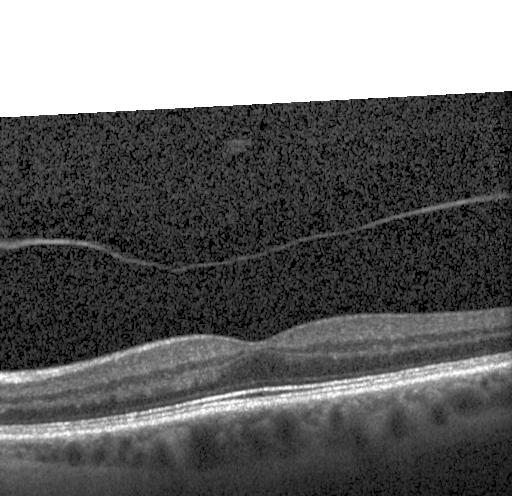

Heidelberg Spectralis OCT system. OCT B-scan. Finding: no evidence of choroidal neovascularization, diabetic macular edema, or drusen.